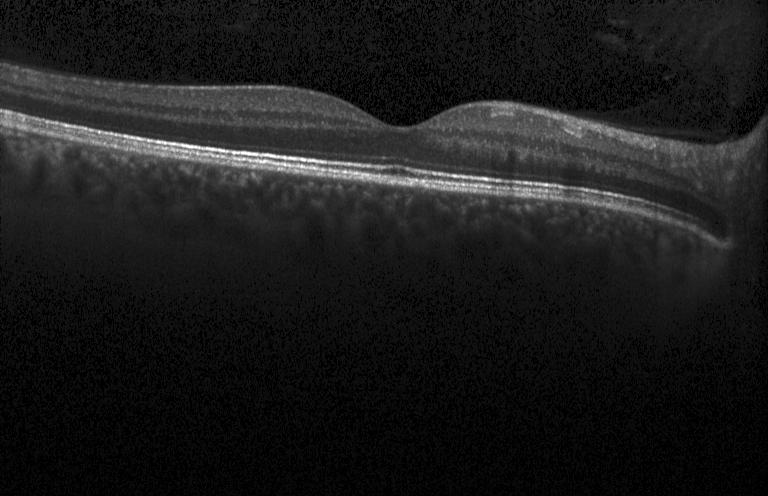

Spectral-domain OCT; optical coherence tomography scan.
No evidence of CNV, DME, or drusen.